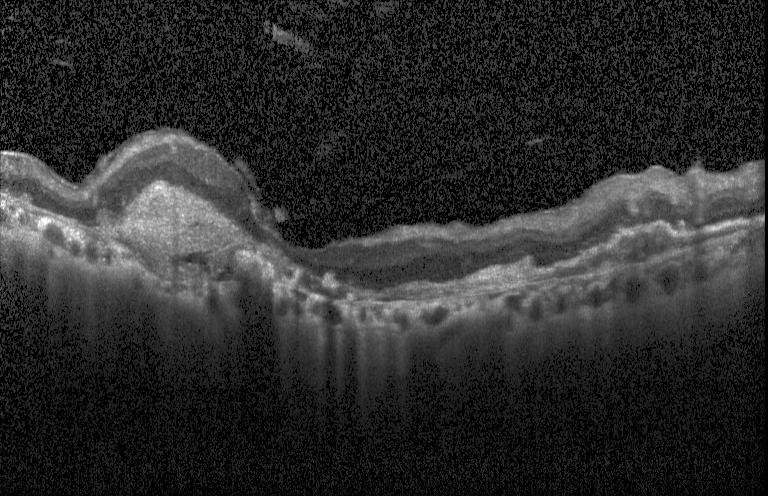
Finding: a choroidal neovascular membrane.